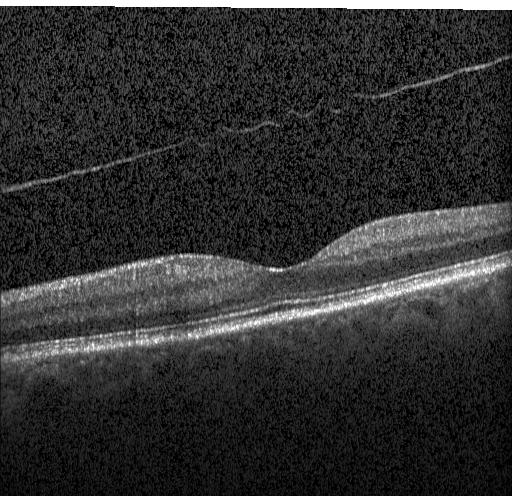 Retinal OCT cross-section showing neither choroidal neovascularization, diabetic macular edema, nor drusen.